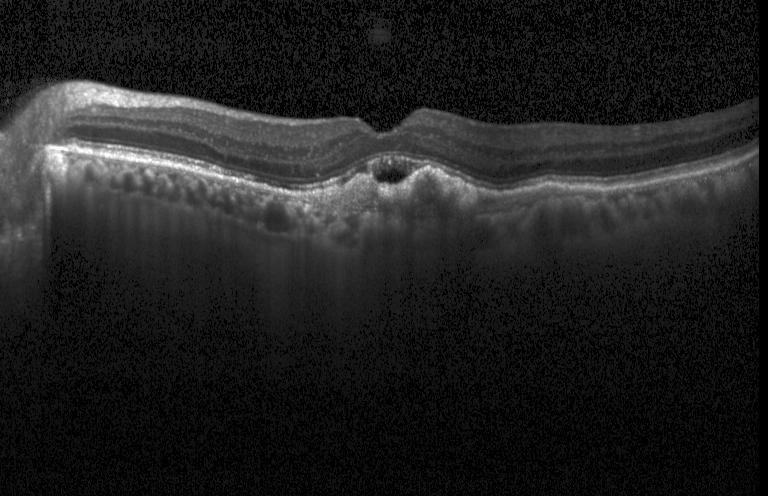

Impression: a choroidal neovascular membrane.